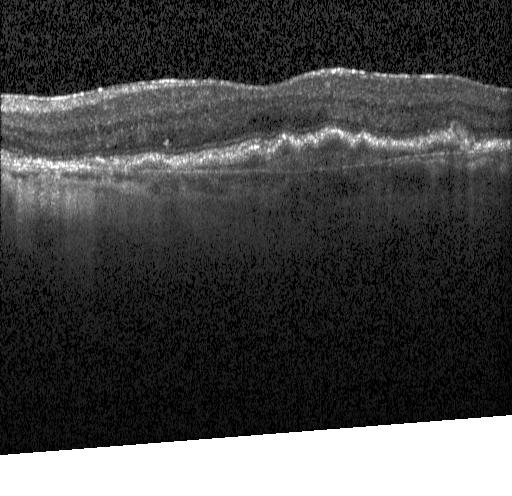

OCT finding: a choroidal neovascular membrane.